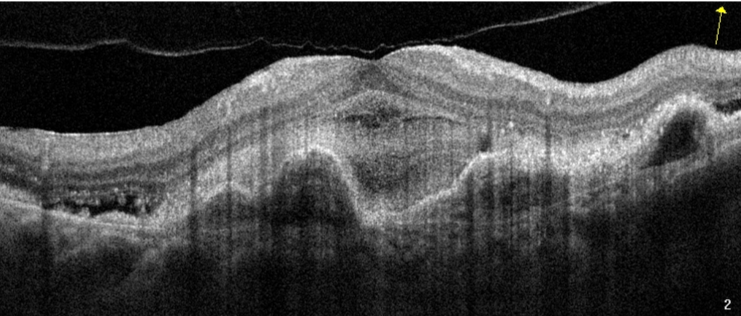

Dx: age-related macular degeneration (AMD).